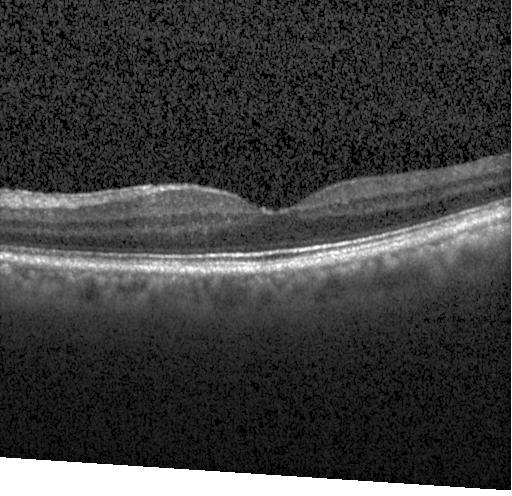
Optical coherence tomography B-scan — Diagnosis: neither choroidal neovascularization, diabetic macular edema, nor drusen.